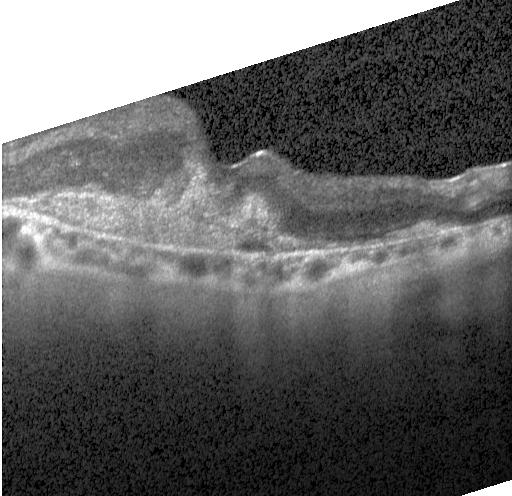 Optical coherence tomography scan
Finding: a choroidal neovascular membrane.